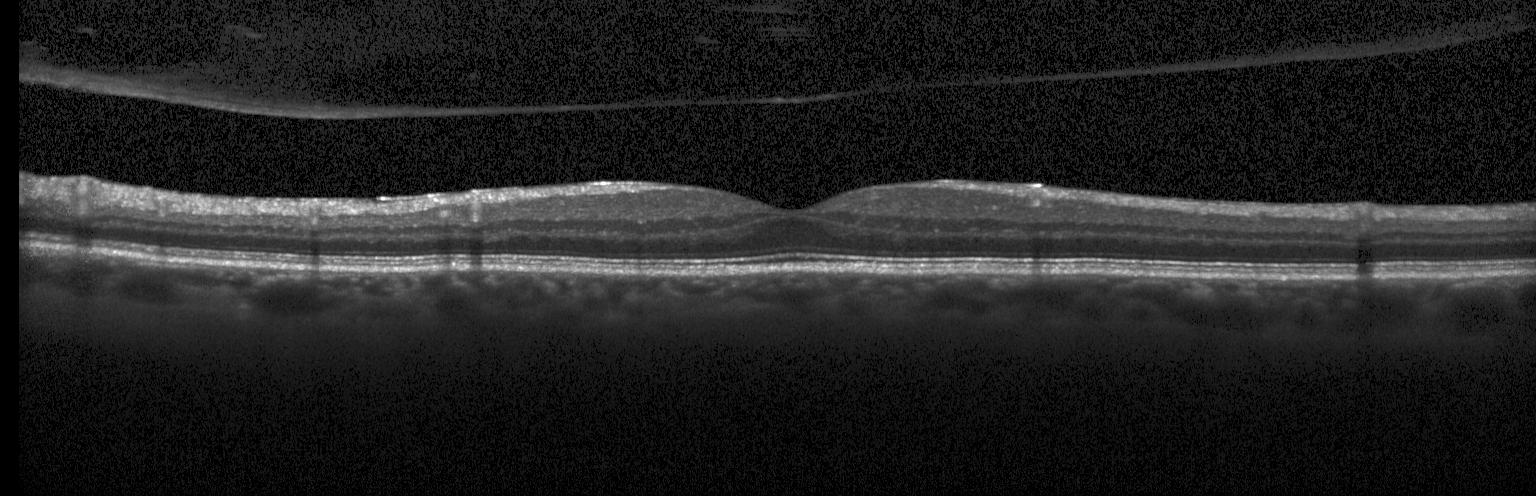
OCT finding: no choroidal neovascularization, diabetic macular edema, or drusen.